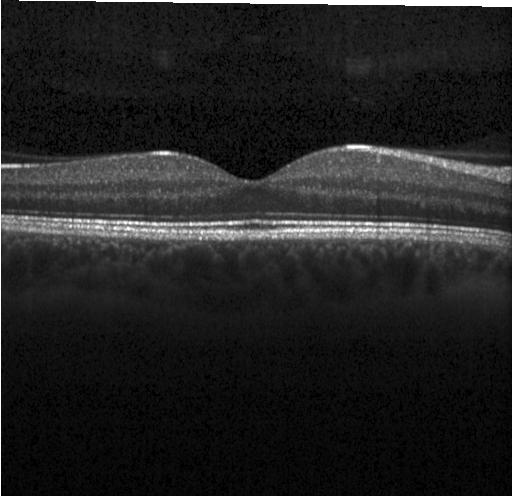 Macular OCT: no choroidal neovascularization, no diabetic macular edema, and no drusen.